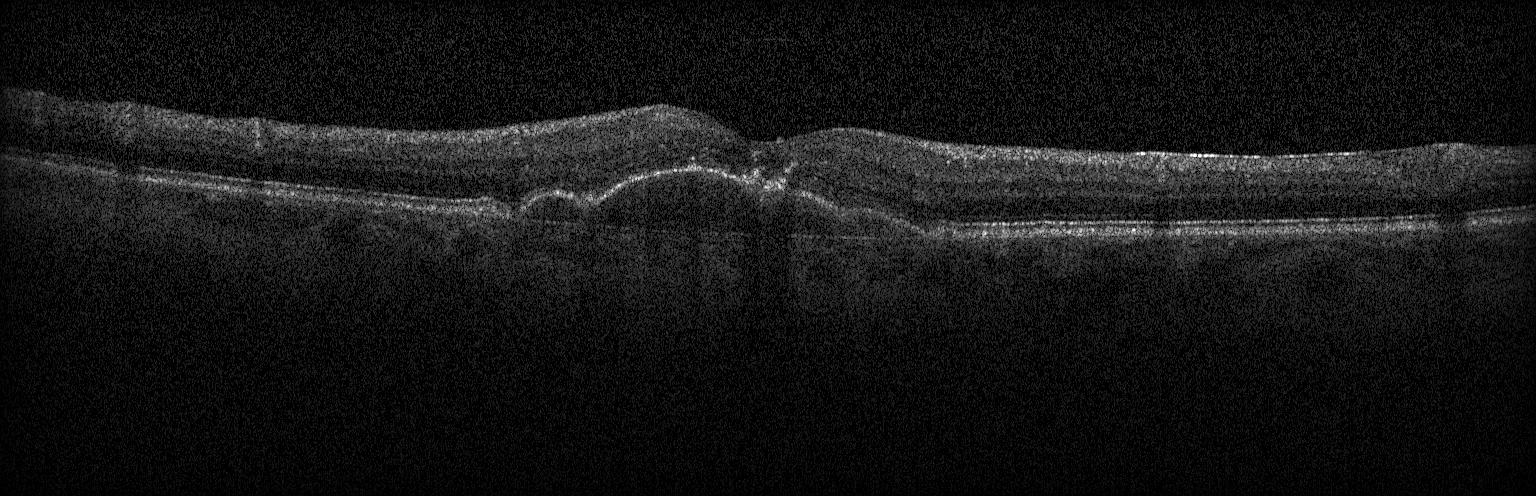

Horizontal scan through the fovea, optical coherence tomography scan.
The scan shows choroidal neovascularization (CNV).